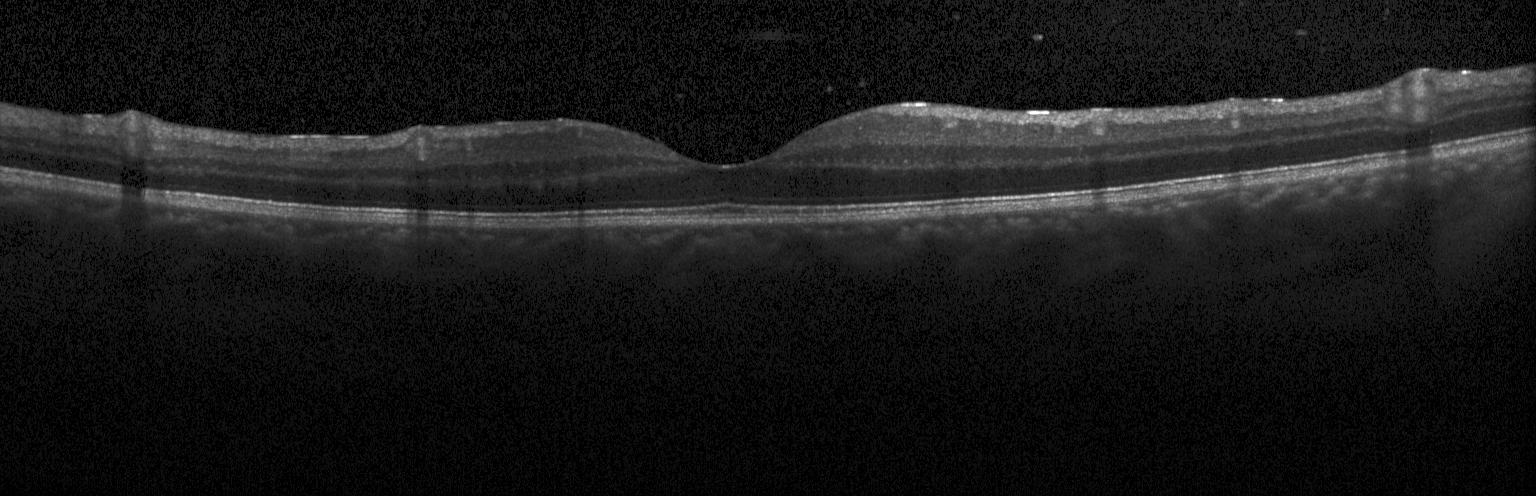 OCT scan showing neither choroidal neovascularization, diabetic macular edema, nor drusen.